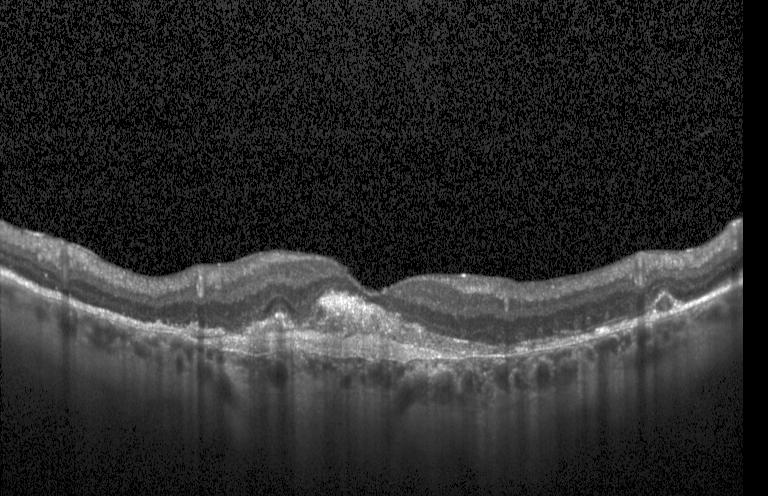
Retinal OCT B-scan. Diagnosis: a choroidal neovascular membrane.